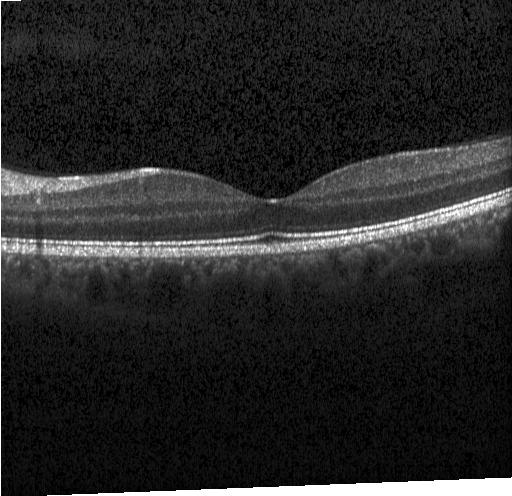

Centered on the fovea, spectral-domain optical coherence tomography, OCT B-scan, acquired on a Heidelberg Spectralis — Macular OCT: no evidence of CNV, DME, or drusen.